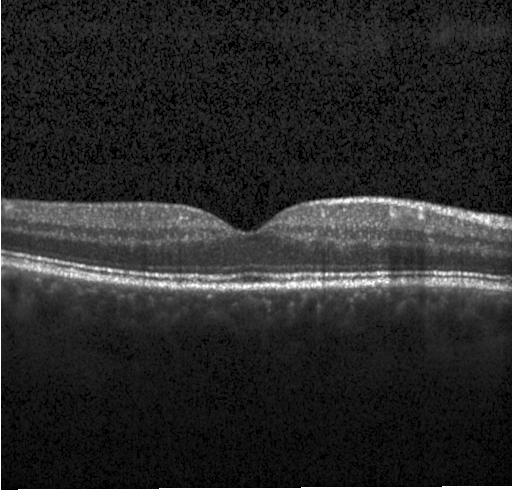

Heidelberg Spectralis OCT system; fovea-centered; optical coherence tomography B-scan; spectral-domain optical coherence tomography. OCT finding: no choroidal neovascularization, diabetic macular edema, or drusen.